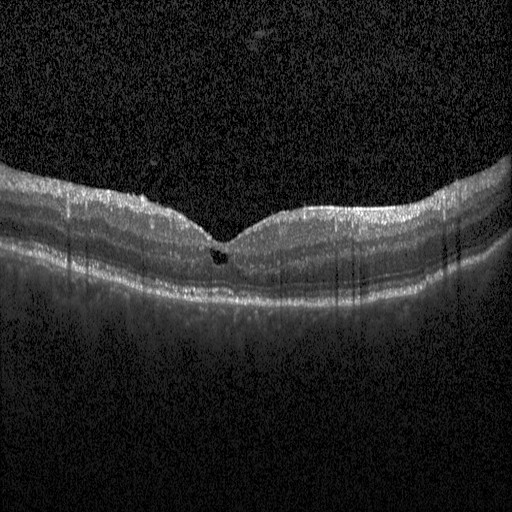 OCT finding: DME.